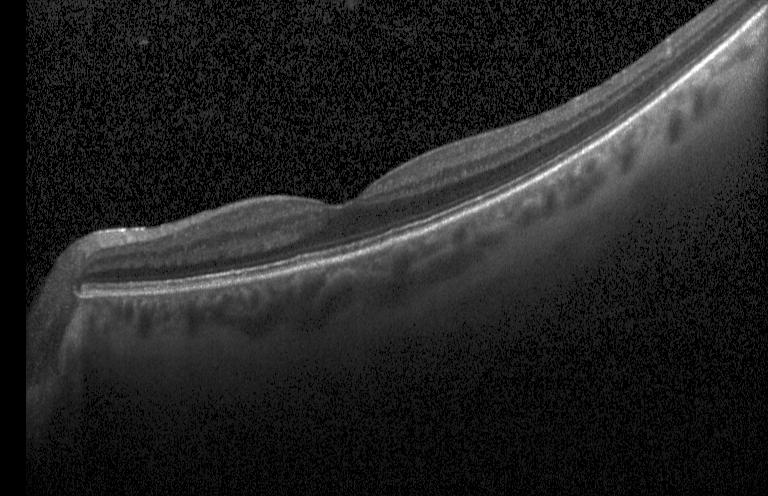
Finding: no evidence of choroidal neovascularization, diabetic macular edema, or drusen.